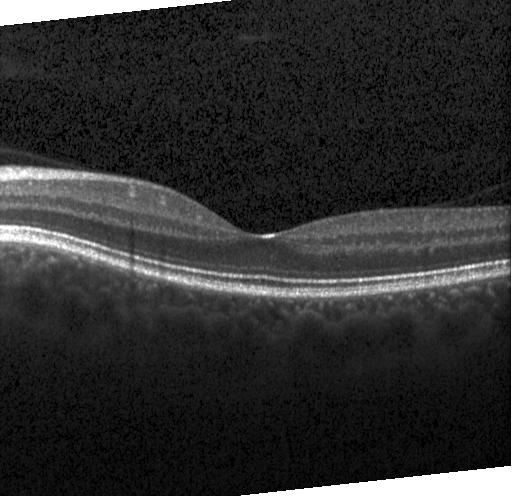
Retinal OCT cross-section — OCT finding: no evidence of CNV, DME, or drusen.